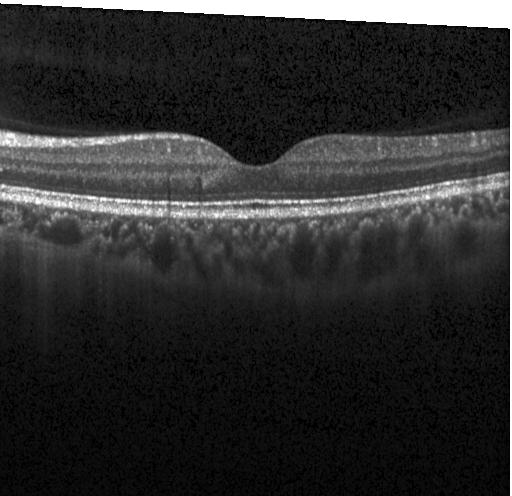 Through the macula, retinal OCT cross-section — This B-scan demonstrates no evidence of CNV, DME, or drusen.